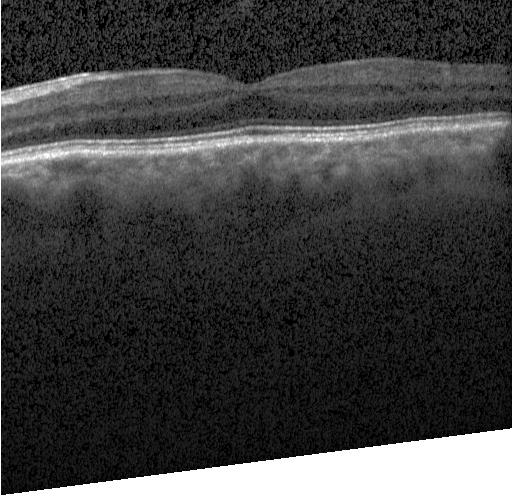

Finding: neither CNV, DME, nor drusen.